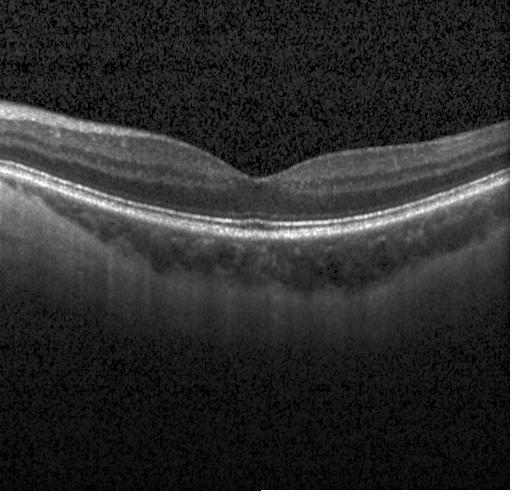 Retinal OCT B-scan. Assessment: no CNV, no DME, and no drusen.